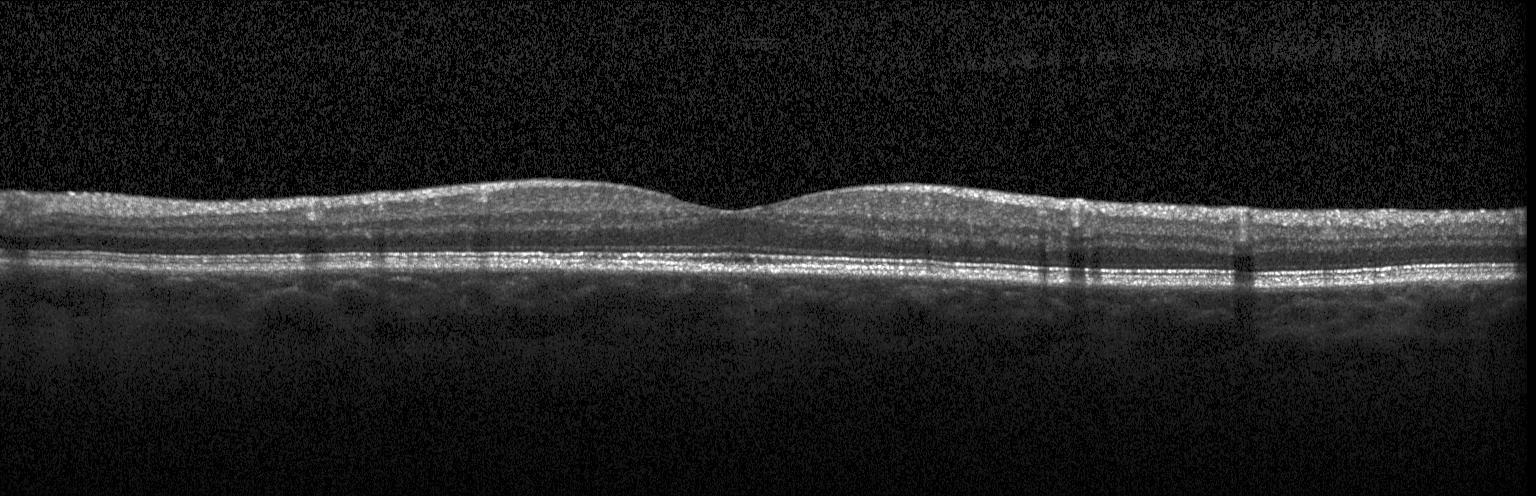

Retinal OCT B-scan, instrument: Heidelberg Spectralis
Impression: neither choroidal neovascularization, diabetic macular edema, nor drusen.